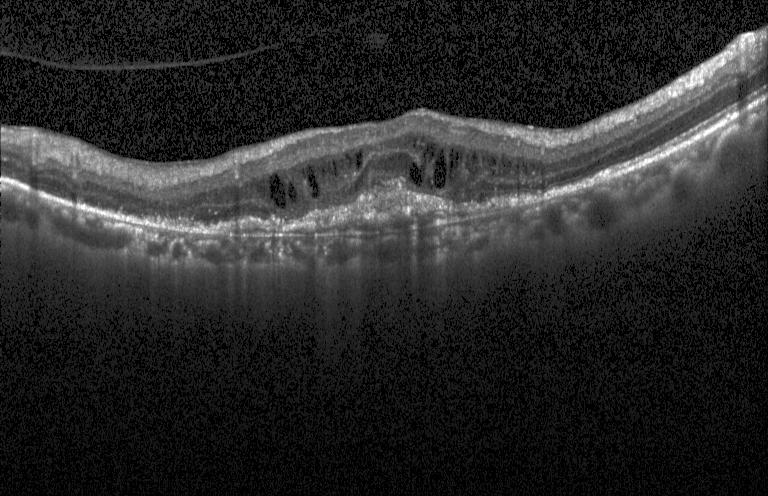 Optical coherence tomography scan
Diagnosis: a choroidal neovascular membrane.